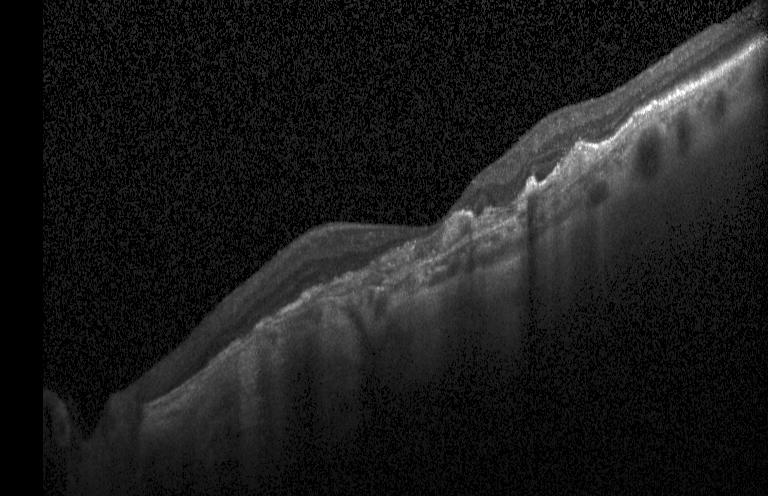

The scan shows a choroidal neovascular membrane.